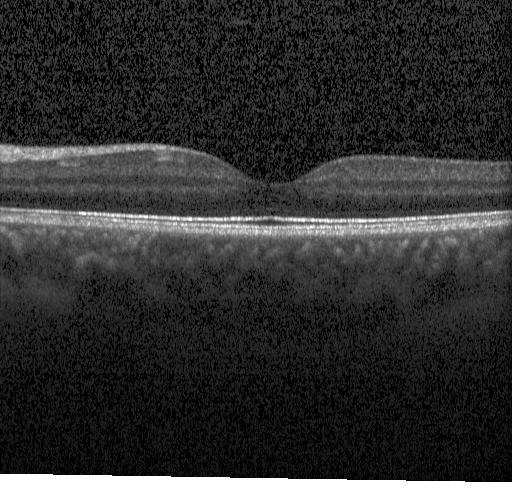

OCT line scan — Neither choroidal neovascularization, diabetic macular edema, nor drusen.